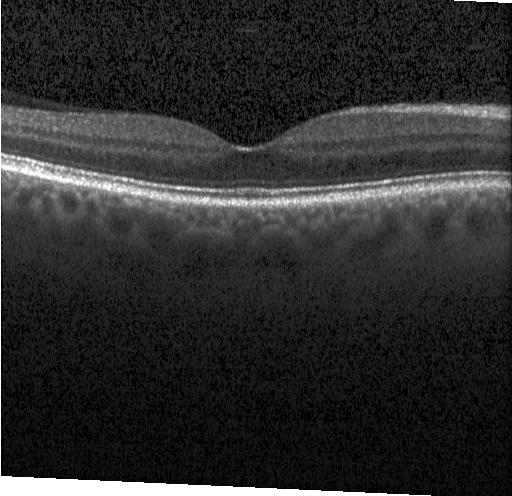 OCT scan showing no CNV, DME, or drusen.